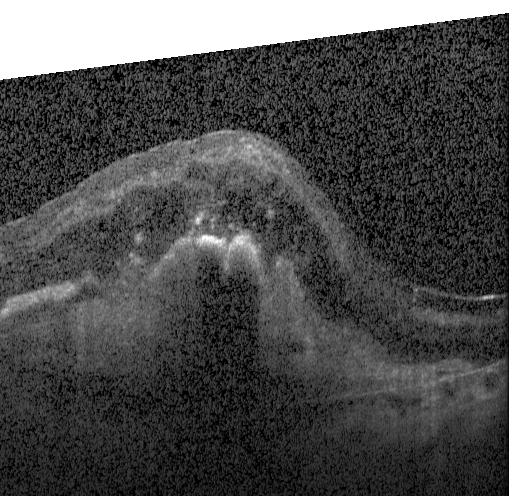

Optical coherence tomography B-scan.
Diagnosis: CNV.